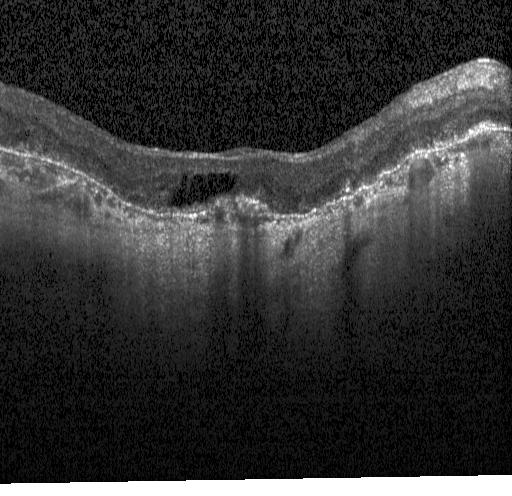

Spectral-domain OCT, optical coherence tomography B-scan.
Impression: a choroidal neovascular membrane.